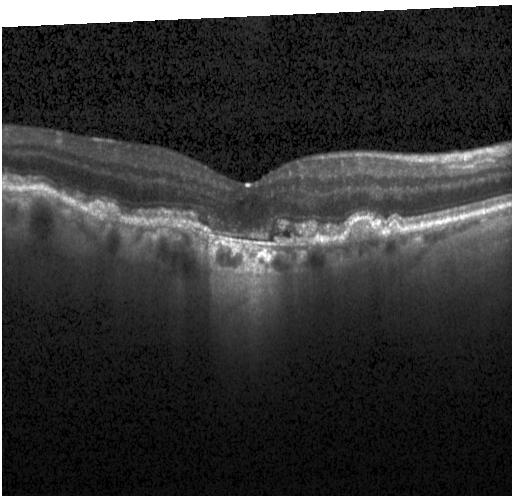

The scan shows a choroidal neovascular membrane.